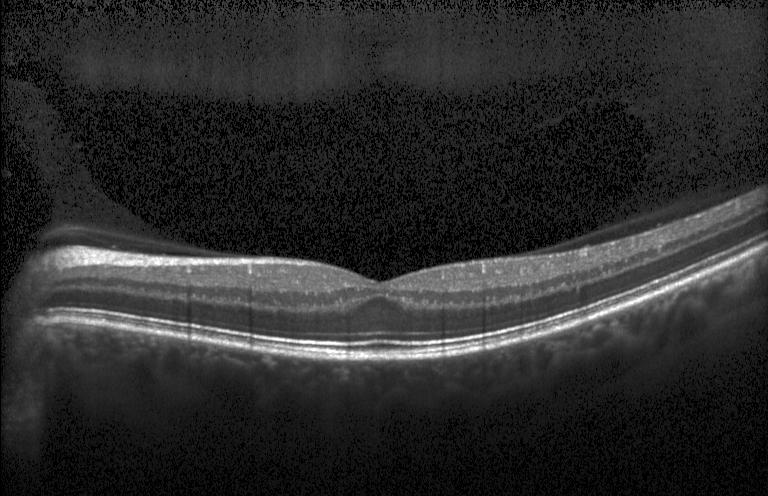

Spectral-domain optical coherence tomography; retinal OCT B-scan; fovea-centered; instrument: Heidelberg Spectralis — The scan shows no evidence of CNV, DME, or drusen.